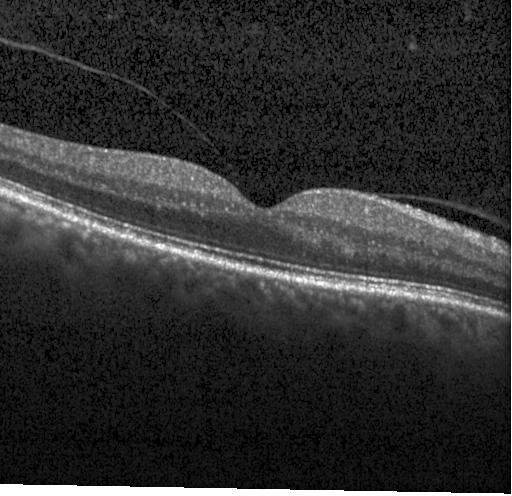
Acquired on a Heidelberg Spectralis · horizontal scan through the fovea · retinal OCT cross-section
The scan shows neither choroidal neovascularization, diabetic macular edema, nor drusen.